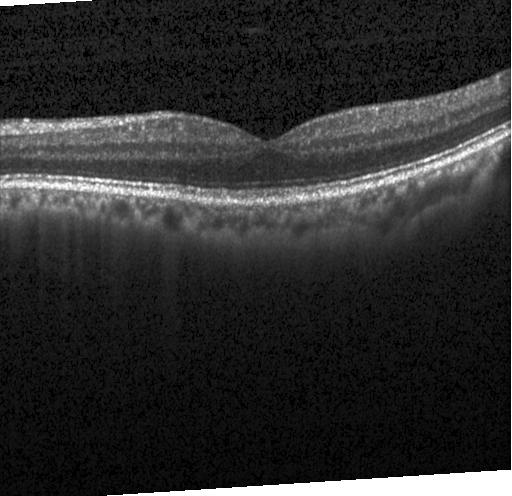 Macular OCT demonstrating no CNV, DME, or drusen.